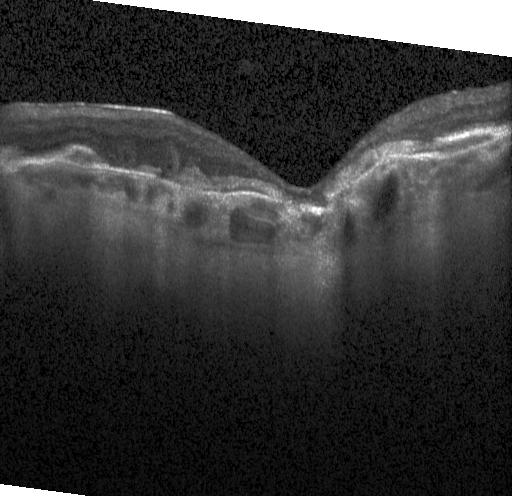 Spectral-domain OCT, retinal OCT cross-section, horizontal scan through the fovea.
Impression: a choroidal neovascular membrane.